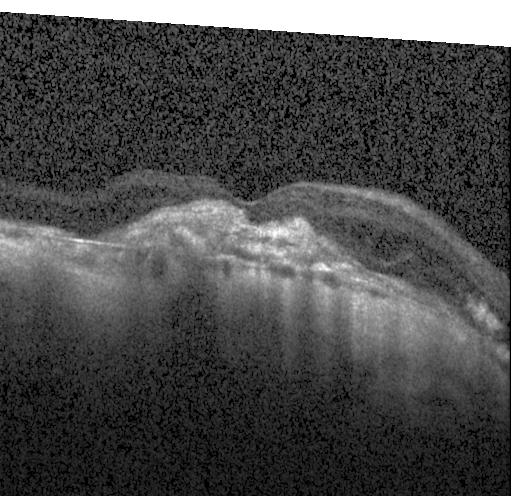
OCT finding: choroidal neovascularization (CNV).